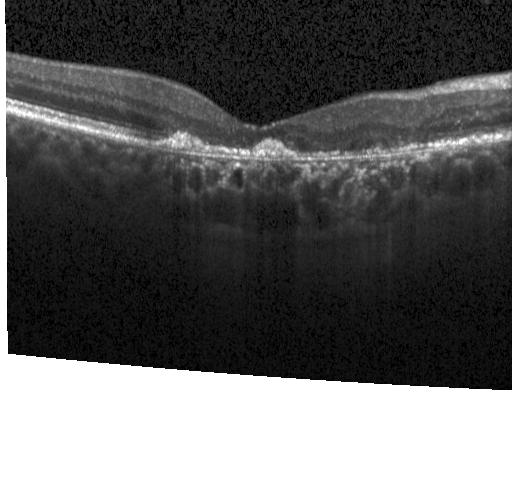
Impression: choroidal neovascularization (CNV).